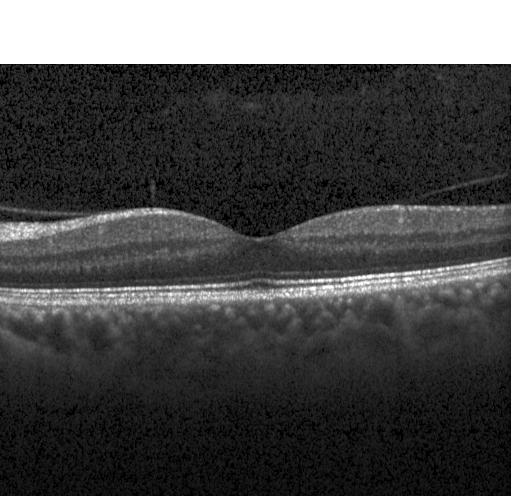 Centered on the fovea. Retinal OCT B-scan. Spectral-domain OCT.
OCT finding: no evidence of CNV, DME, or drusen.